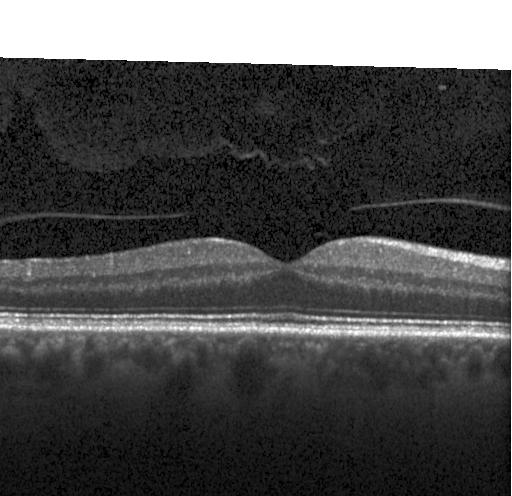

Retinal OCT cross-section.
No evidence of CNV, DME, or drusen.